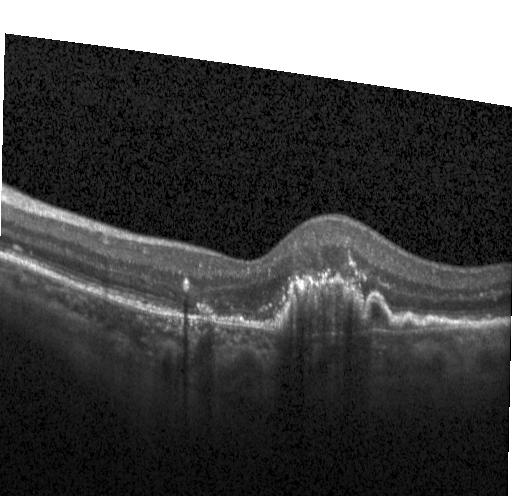

OCT finding: CNV.